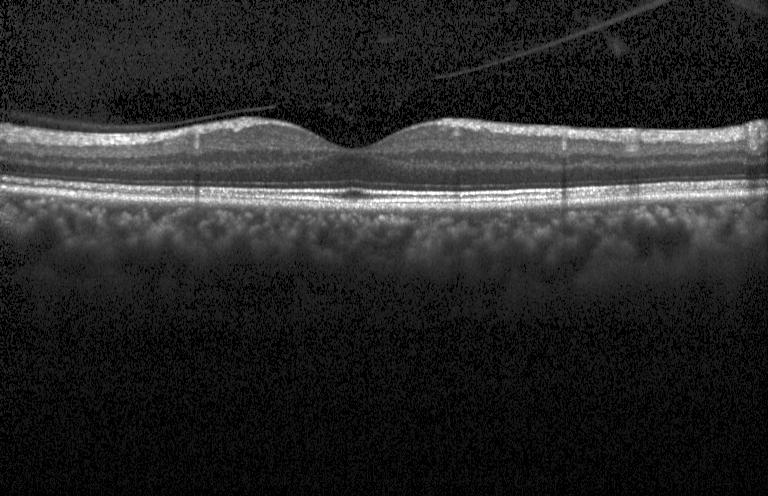
OCT line scan — Assessment: no choroidal neovascularization, diabetic macular edema, or drusen.